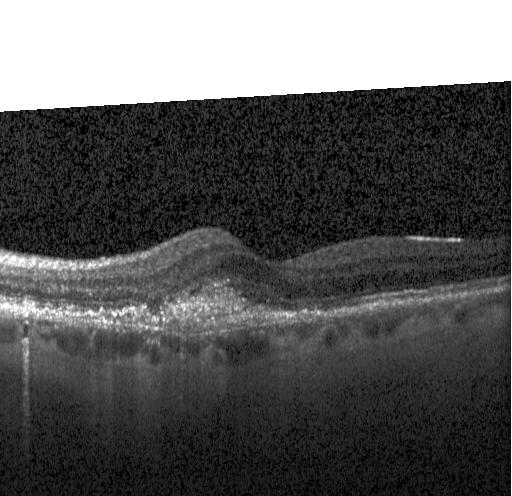
Optical coherence tomography scan · centered on the fovea · Heidelberg Spectralis. OCT finding: choroidal neovascularization.